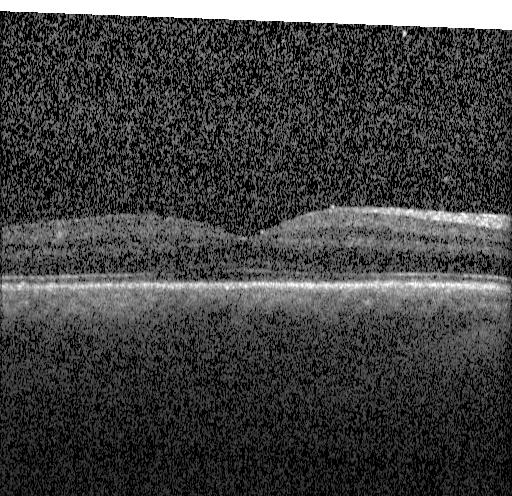
Instrument: Heidelberg Spectralis; SD-OCT; OCT B-scan; centered on the fovea.
OCT finding: no choroidal neovascularization, no diabetic macular edema, and no drusen.